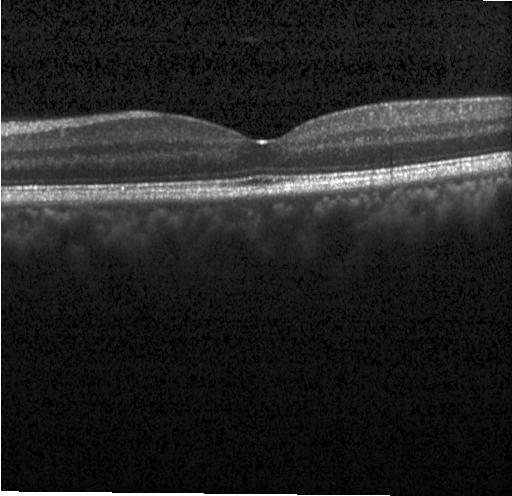

Retinal OCT cross-section, spectral-domain optical coherence tomography. Assessment: no choroidal neovascularization, diabetic macular edema, or drusen.